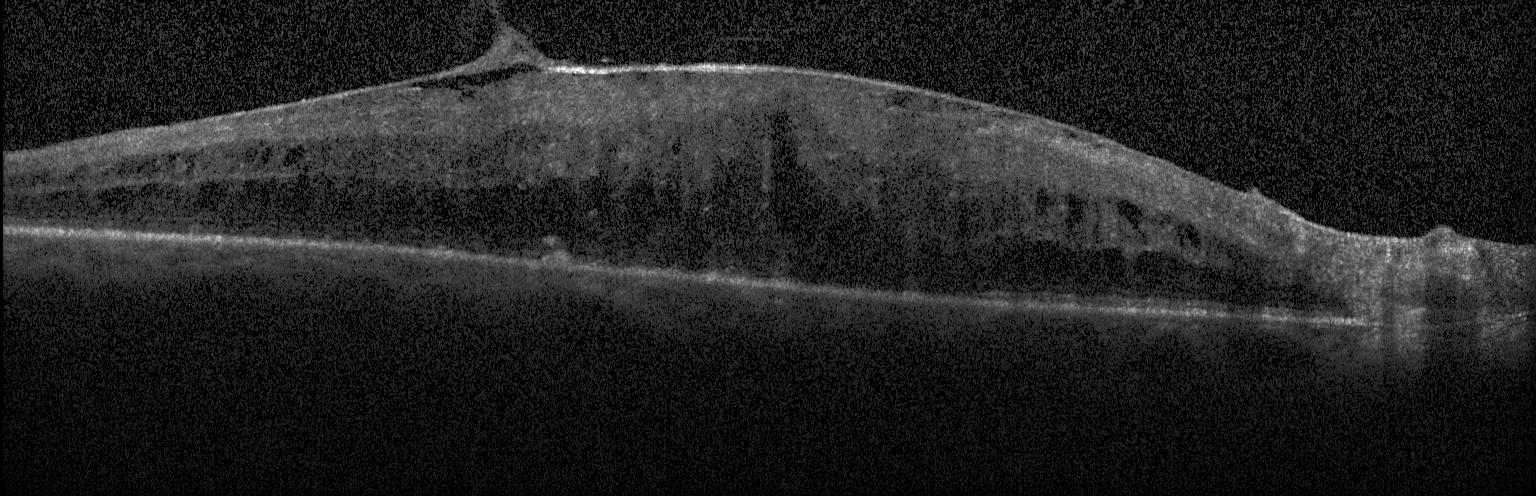 Instrument: Heidelberg Spectralis · retinal OCT cross-section.
Diagnosis: diabetic macular edema.